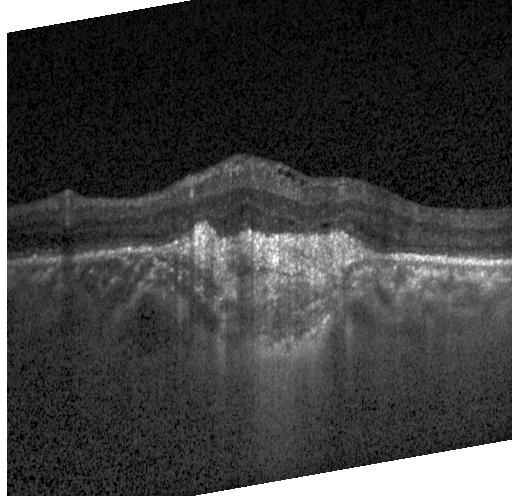
OCT scan showing CNV.